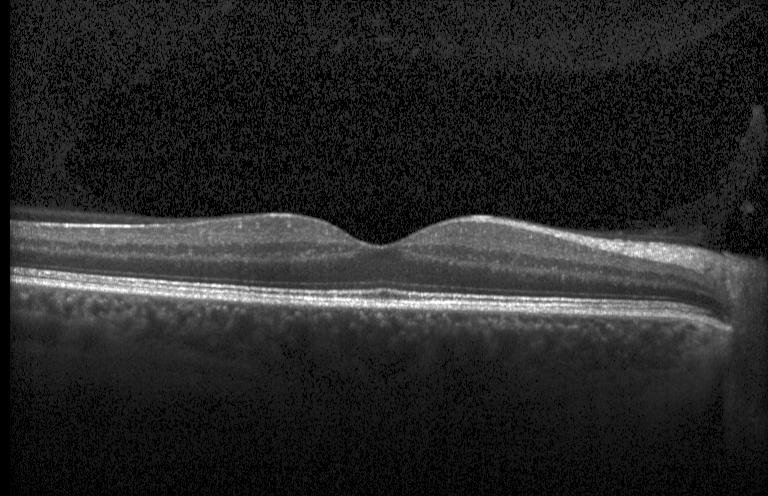

Optical coherence tomography B-scan; SD-OCT; instrument: Heidelberg Spectralis
Impression: no evidence of choroidal neovascularization, diabetic macular edema, or drusen.